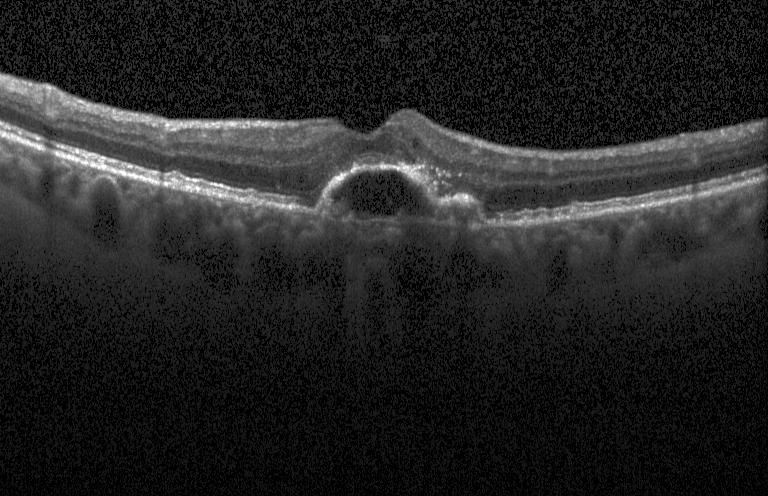

Assessment: a choroidal neovascular membrane.